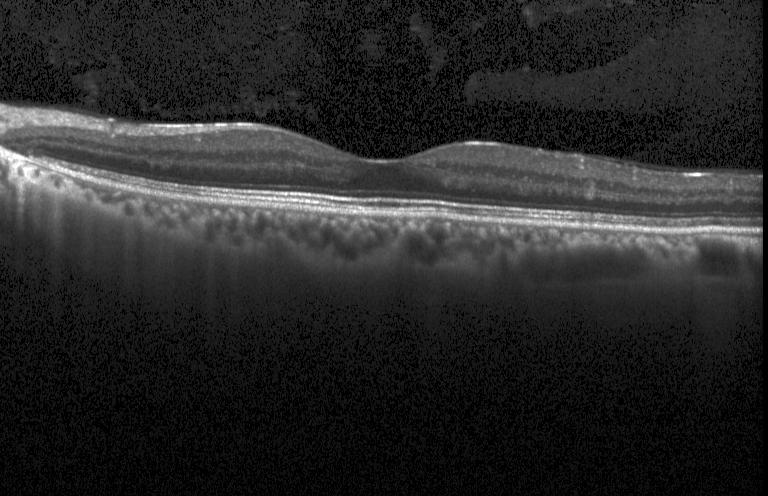 Acquired on a Heidelberg Spectralis; optical coherence tomography scan.
Assessment: no choroidal neovascularization, no diabetic macular edema, and no drusen.